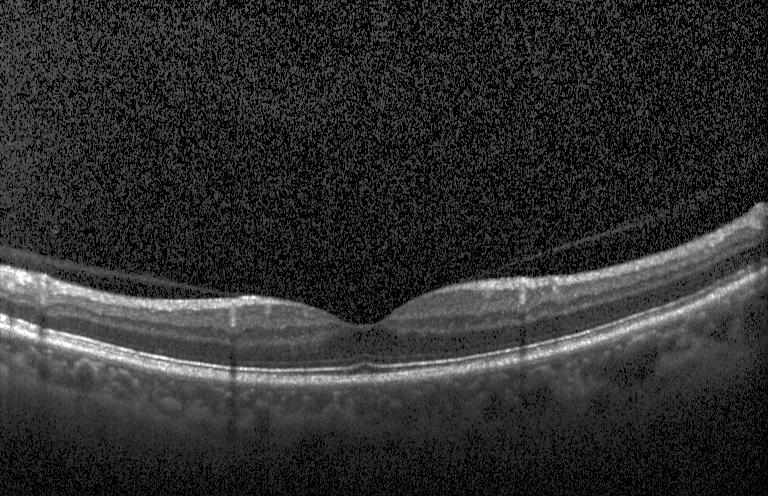 Impression: no evidence of CNV, DME, or drusen.